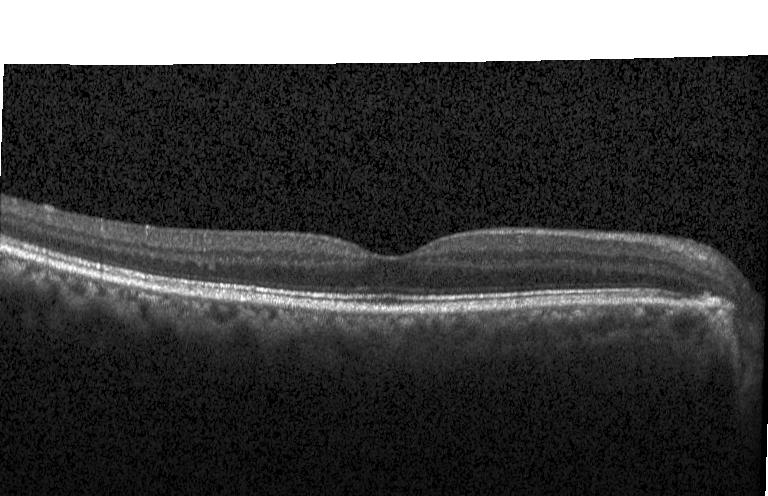 Macular scan · optical coherence tomography scan — Impression: no choroidal neovascularization, diabetic macular edema, or drusen.